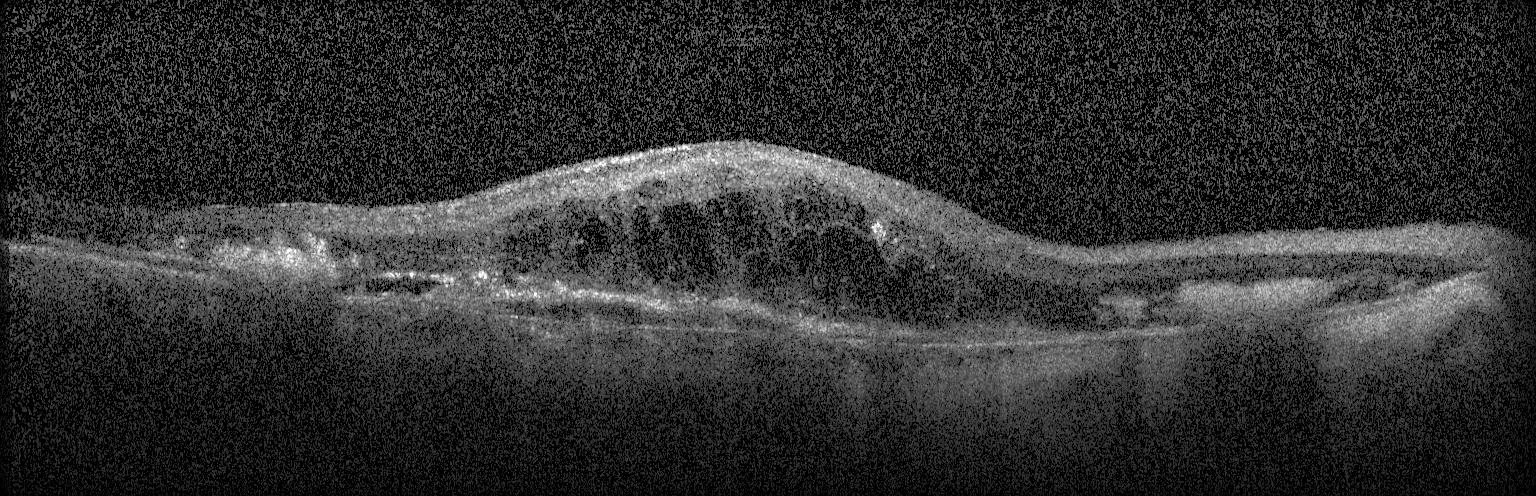 SD-OCT. Optical coherence tomography B-scan
Macular OCT: choroidal neovascularization.